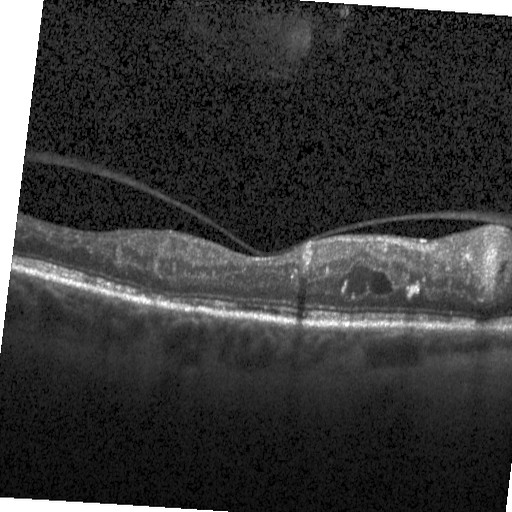
OCT finding: diabetic macular edema.